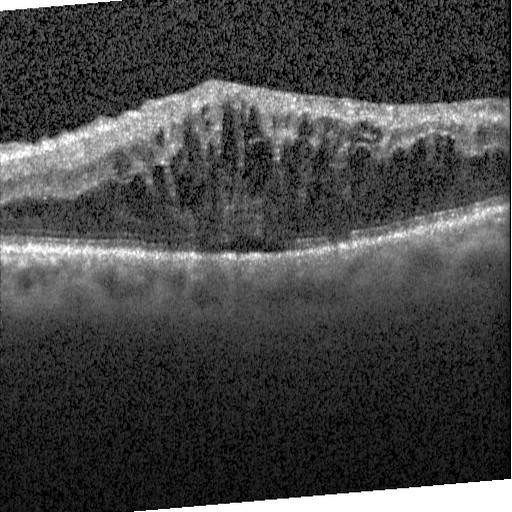 Instrument: Heidelberg Spectralis, spectral-domain optical coherence tomography, fovea-centered, retinal OCT B-scan.
Assessment: diabetic macular edema (DME).